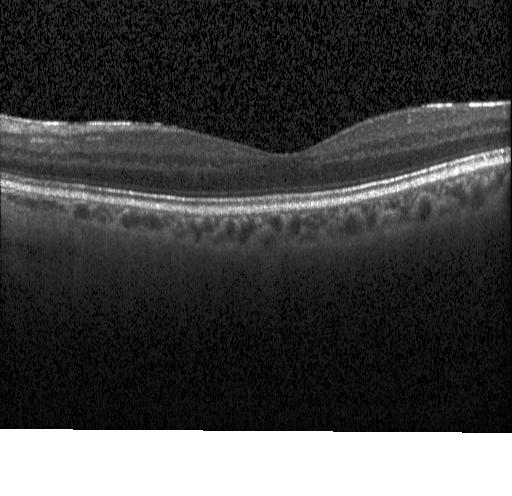 Retinal OCT B-scan, Heidelberg Spectralis OCT system — Diagnosis: no choroidal neovascularization, diabetic macular edema, or drusen.